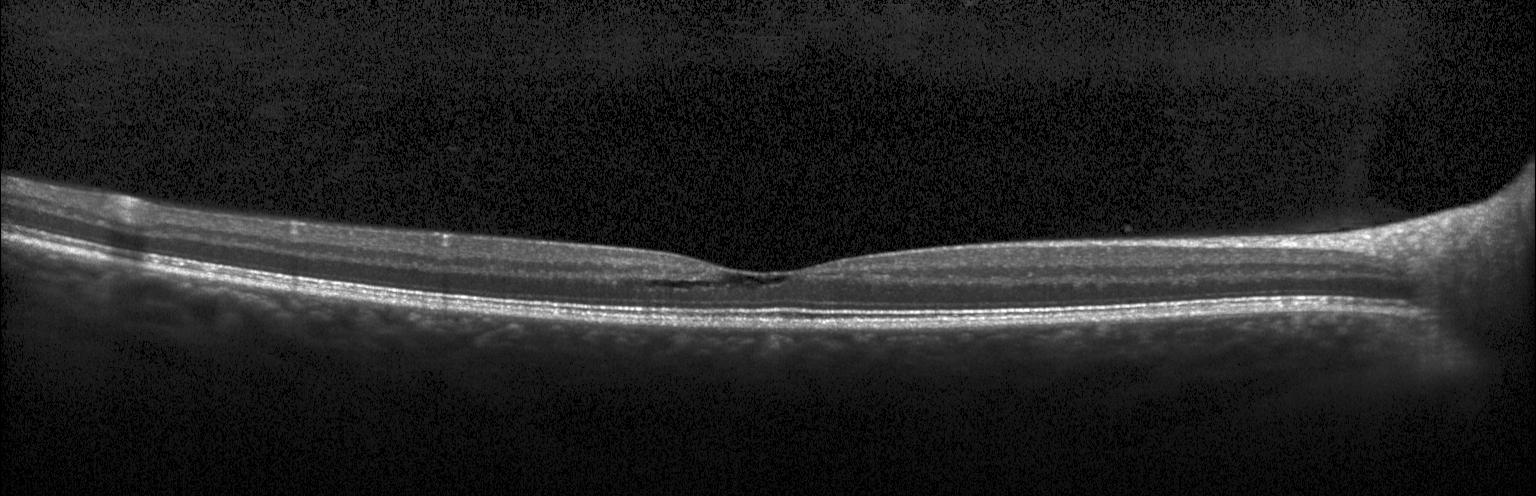
Retinal OCT cross-section · spectral-domain OCT
Impression: DME.